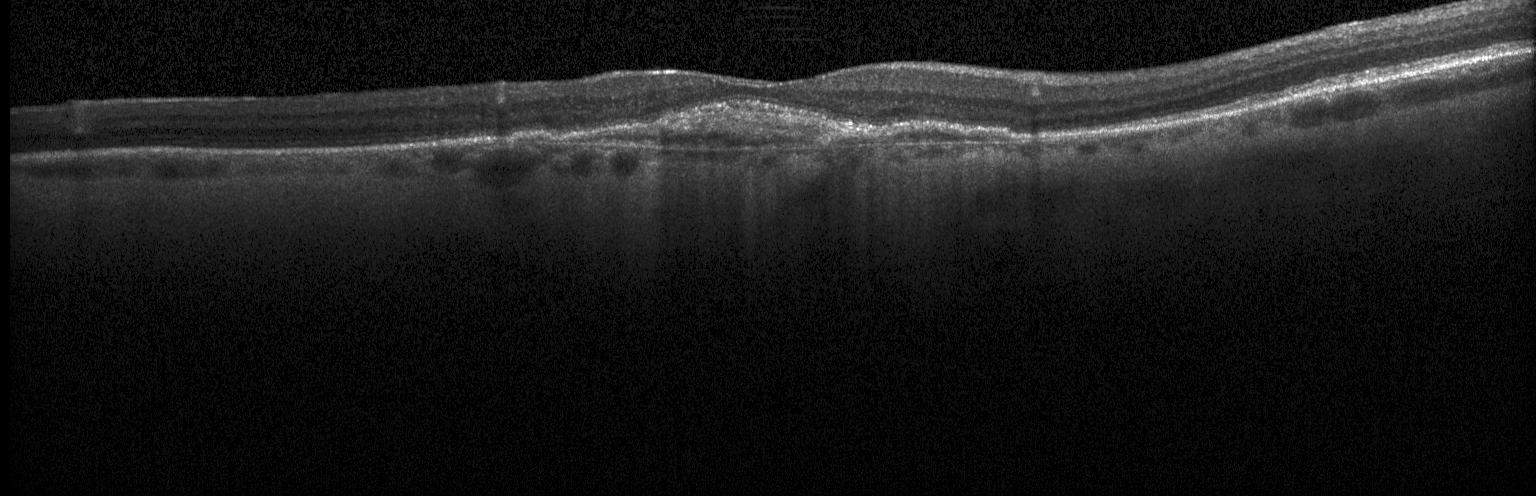 Spectral-domain OCT B-scan: choroidal neovascularization.